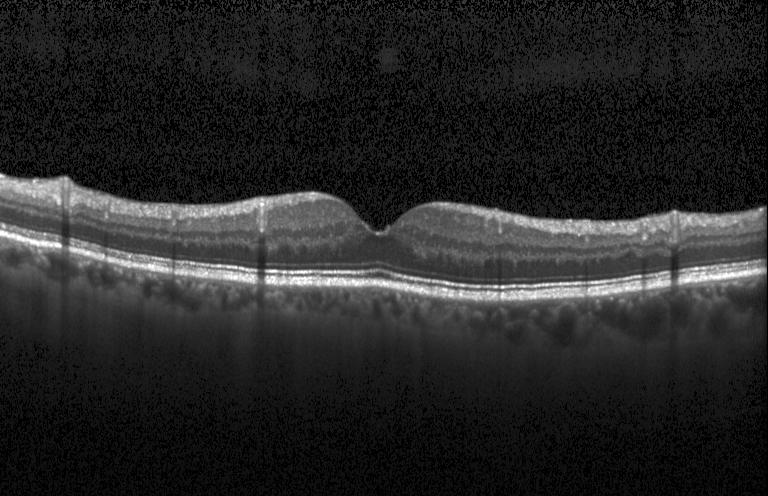
Heidelberg Spectralis OCT system · SD-OCT · retinal OCT B-scan · through the macula. OCT finding: no evidence of choroidal neovascularization, diabetic macular edema, or drusen.